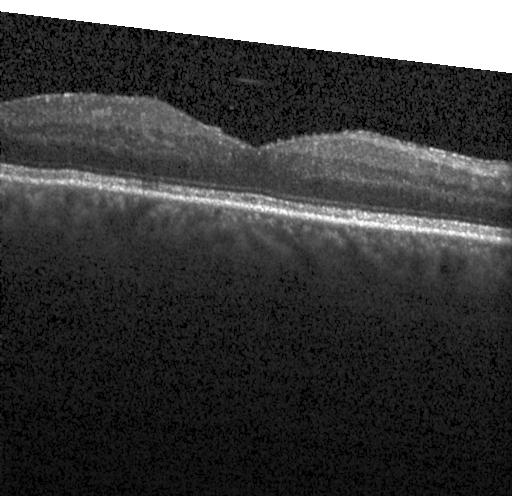 No choroidal neovascularization, diabetic macular edema, or drusen.